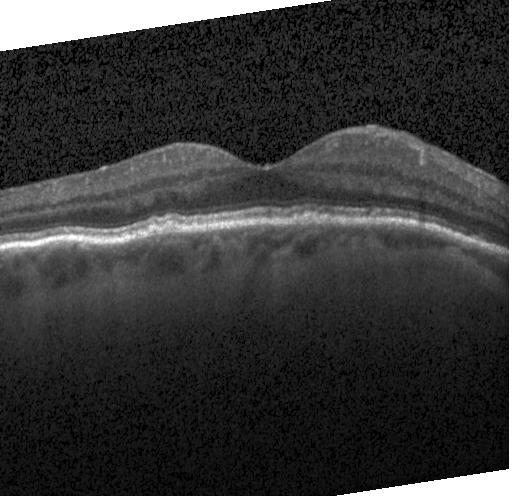
Retinal OCT cross-section showing drusen.